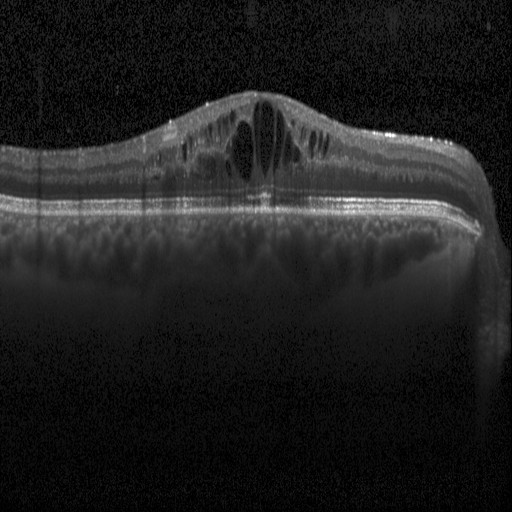 Impression: diabetic macular edema (DME).